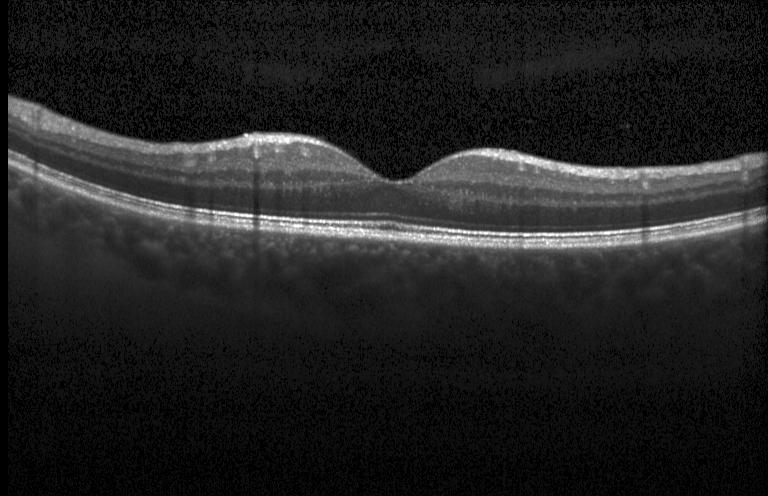 Acquired on a Heidelberg Spectralis, retinal OCT B-scan, centered on the fovea
Diagnosis: no choroidal neovascularization, diabetic macular edema, or drusen.